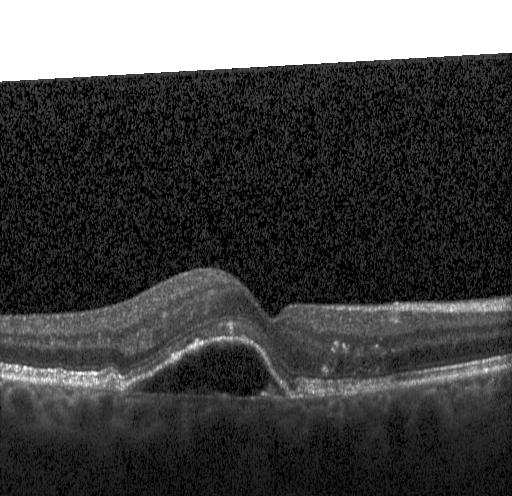 Macular scan. Acquired on a Heidelberg Spectralis. Optical coherence tomography scan. SD-OCT.
Diagnosis: choroidal neovascularization (CNV).